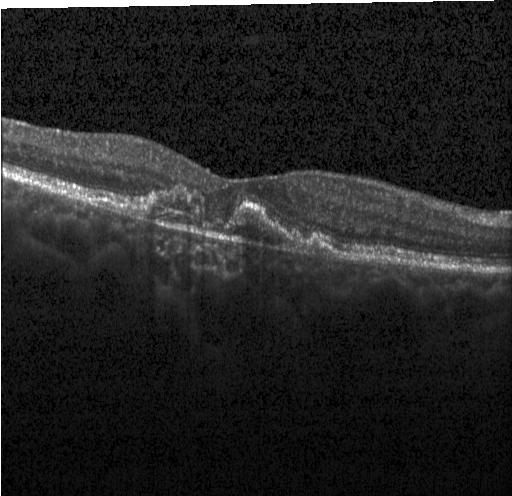
Diagnosis: choroidal neovascularization (CNV).